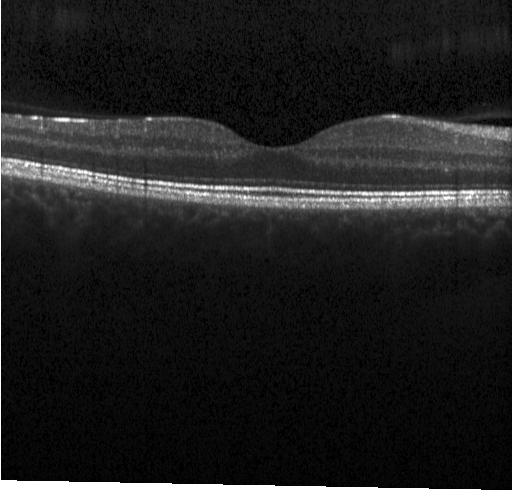
Macular OCT: no choroidal neovascularization, no diabetic macular edema, and no drusen.